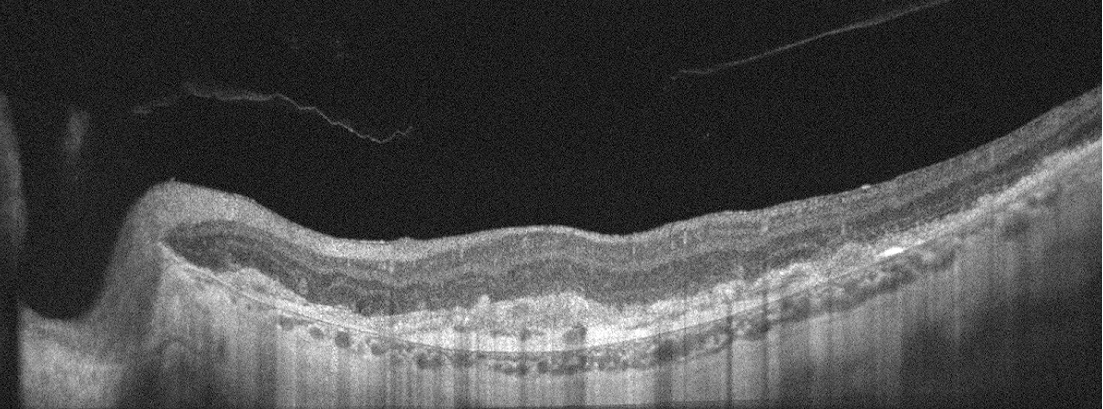

Fovea-centered · retinal OCT cross-section.
Assessment: age-related macular degeneration.